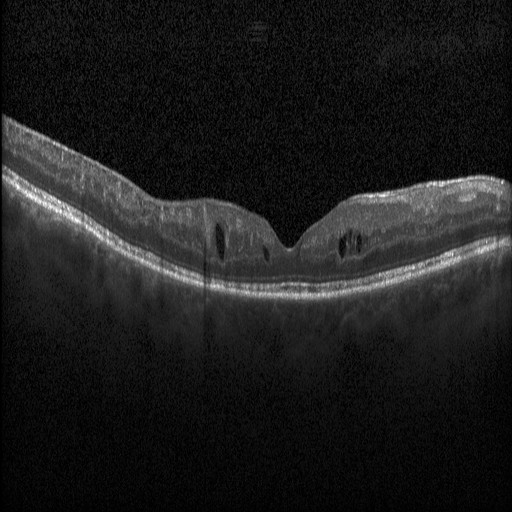

SD-OCT, optical coherence tomography scan.
Finding: DME.